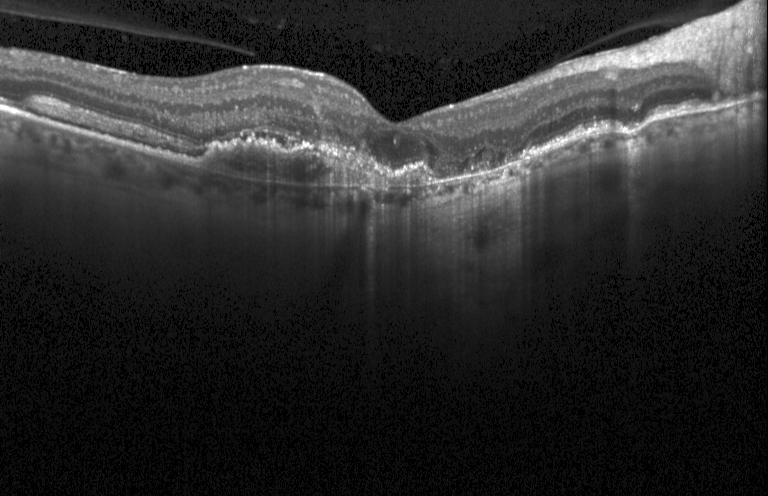
This B-scan demonstrates choroidal neovascularization (CNV).